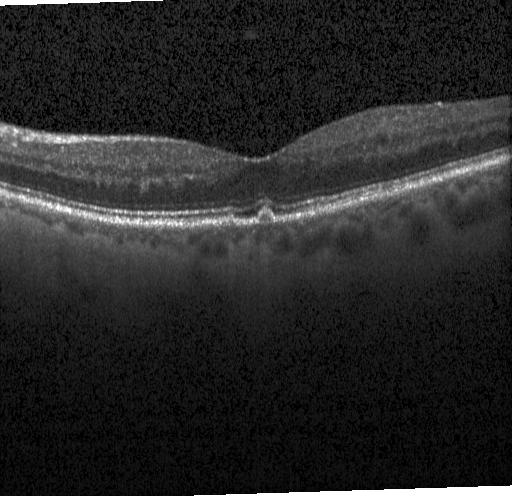

OCT scan showing drusen.